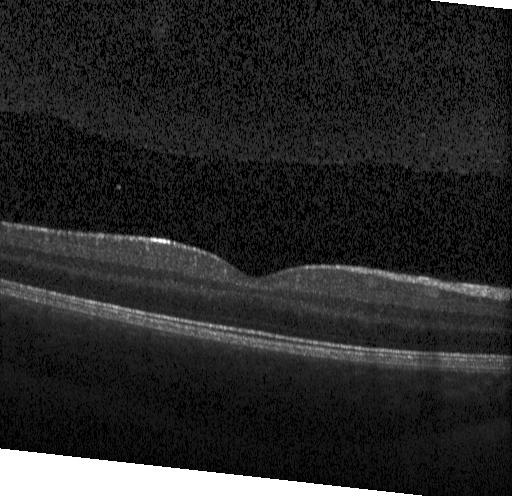 Retinal OCT cross-section
Impression: no CNV, no DME, and no drusen.